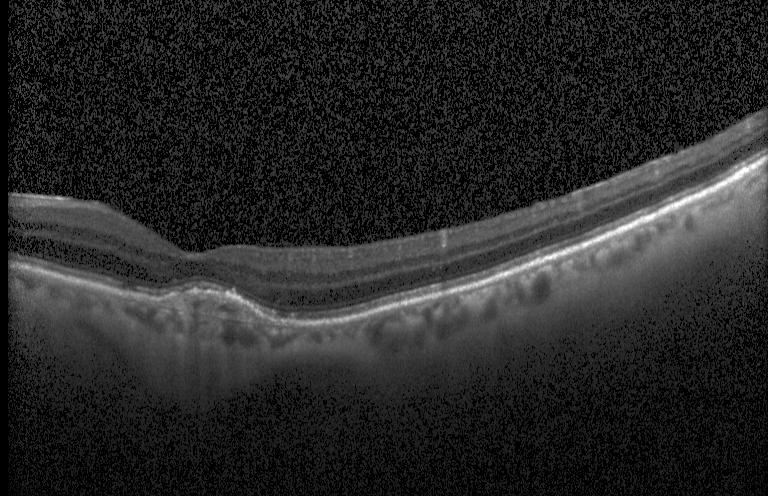
Impression: a choroidal neovascular membrane.